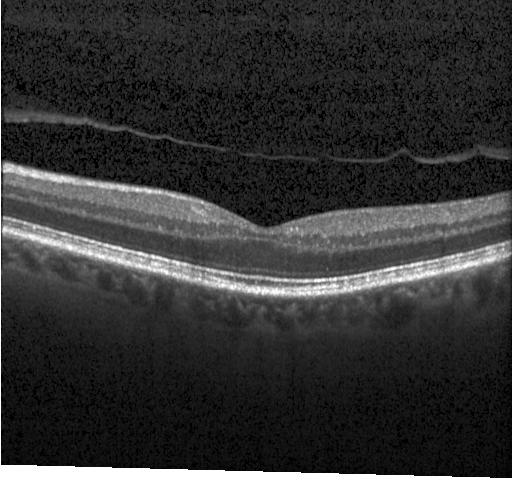
Instrument: Heidelberg Spectralis; centered on the fovea; spectral-domain OCT; OCT B-scan. Impression: neither CNV, DME, nor drusen.